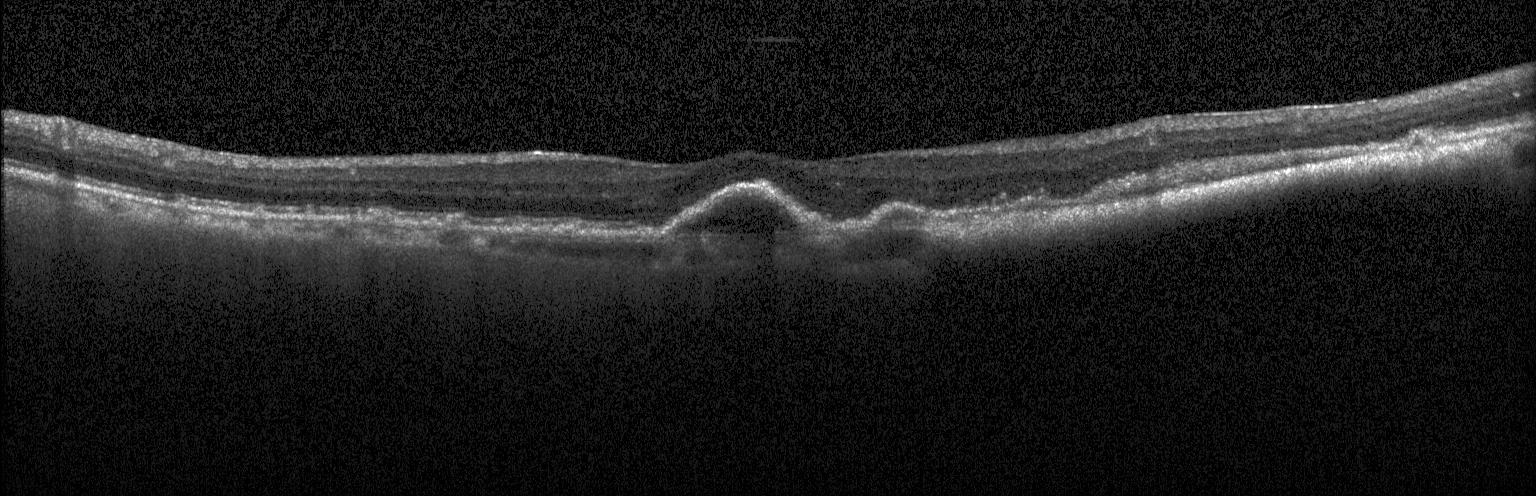

Heidelberg Spectralis; macular scan; SD-OCT; OCT line scan.
Dx: choroidal neovascularization (CNV).